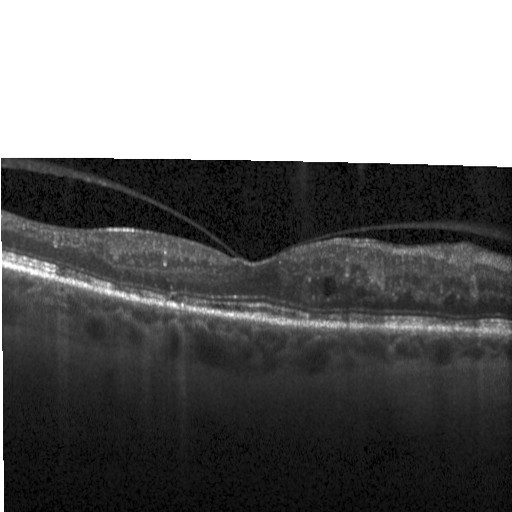
Impression: diabetic macular edema (DME).